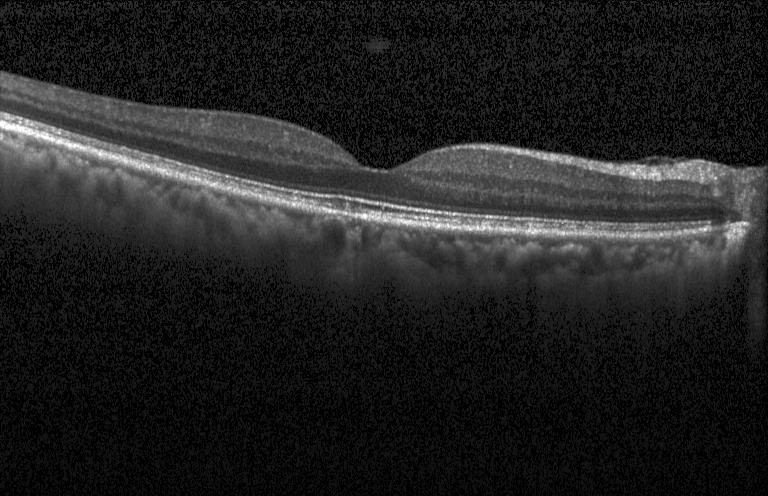

Spectral-domain OCT; retinal OCT B-scan. The scan shows no choroidal neovascularization, no diabetic macular edema, and no drusen.